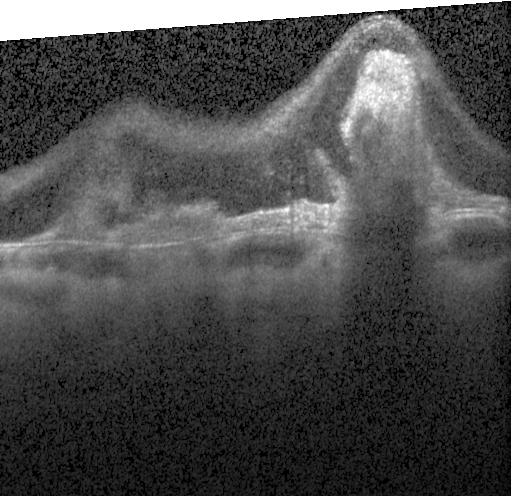 Horizontal scan through the fovea; spectral-domain optical coherence tomography; instrument: Heidelberg Spectralis; OCT B-scan — The scan shows a choroidal neovascular membrane.